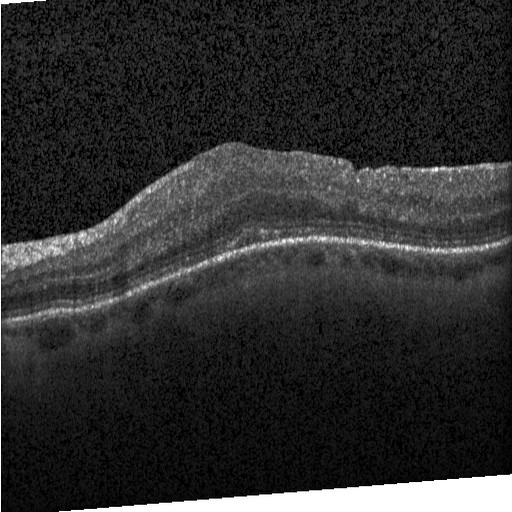 DME.